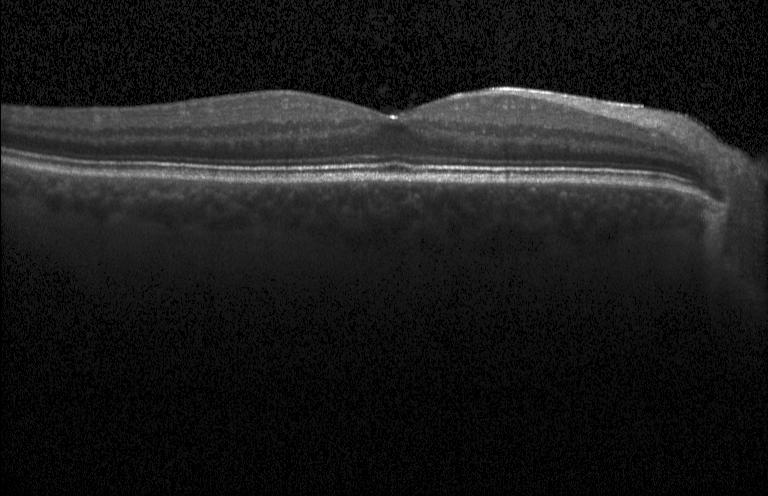
Dx: no choroidal neovascularization, no diabetic macular edema, and no drusen.